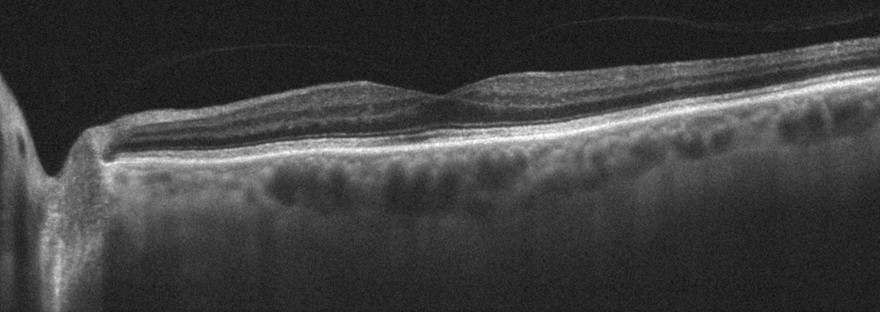 No evidence of AMD, DME, ERM, RAO, RVO, or VID.